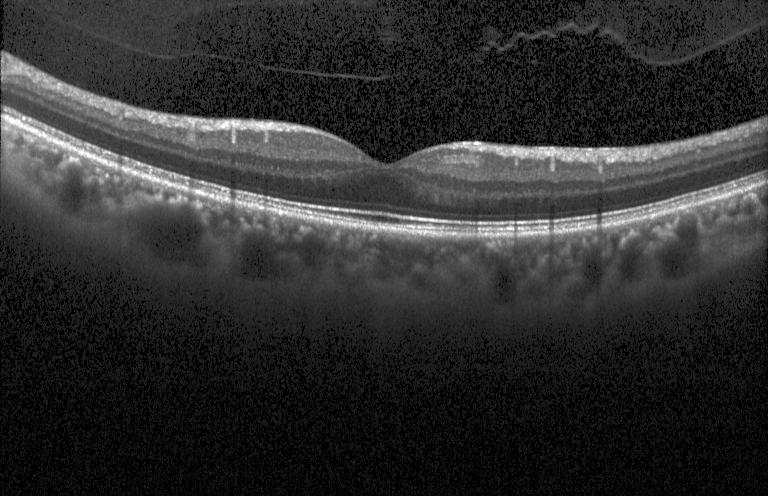 OCT B-scan. Impression: neither CNV, DME, nor drusen.